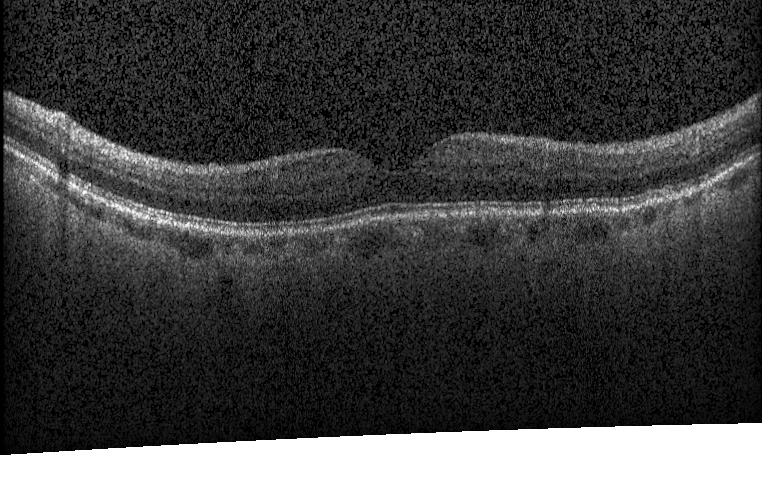

Macular OCT: no choroidal neovascularization, no diabetic macular edema, and no drusen.